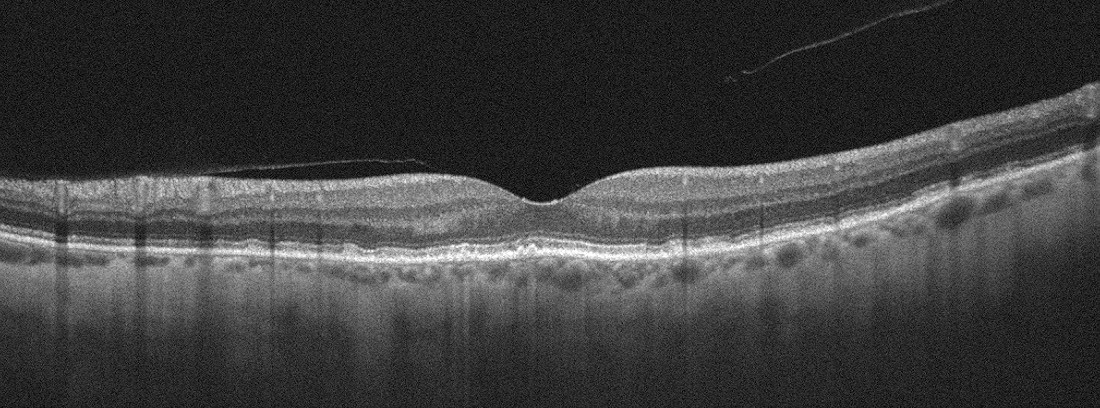
OCT line scan. OCT finding: age-related macular degeneration (AMD).